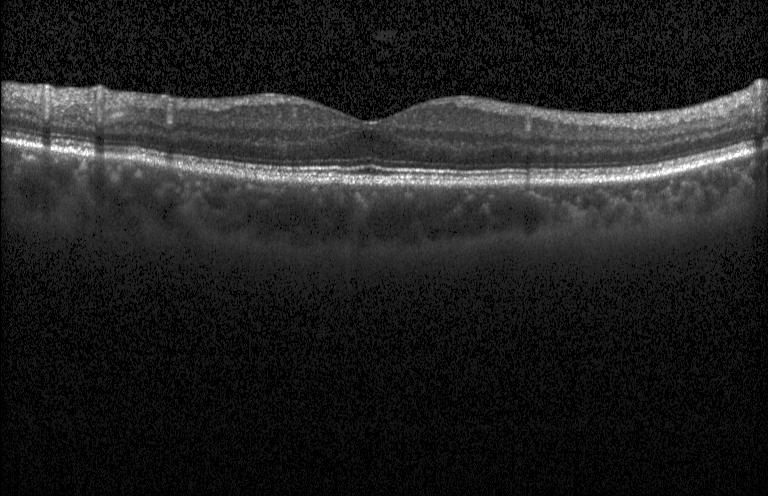

OCT line scan; acquired on a Heidelberg Spectralis
Finding: no evidence of choroidal neovascularization, diabetic macular edema, or drusen.